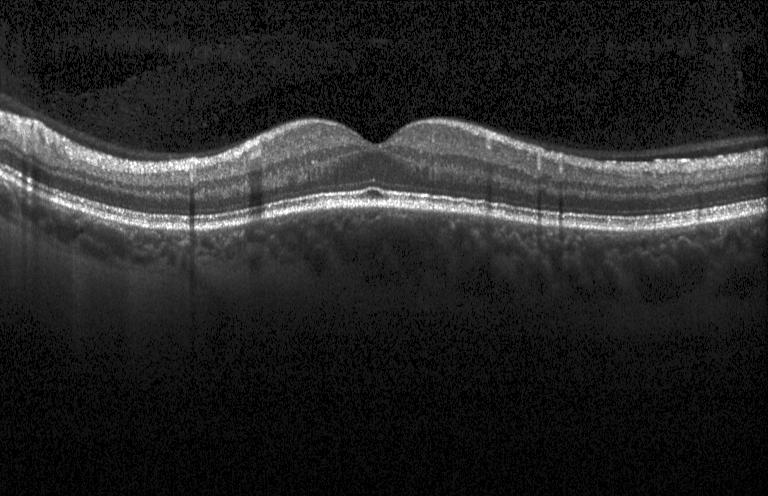

OCT B-scan — Finding: no choroidal neovascularization, no diabetic macular edema, and no drusen.